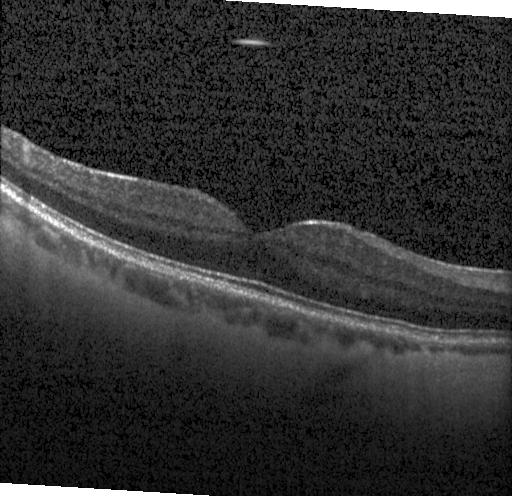

Retinal OCT cross-section showing no choroidal neovascularization, no diabetic macular edema, and no drusen.